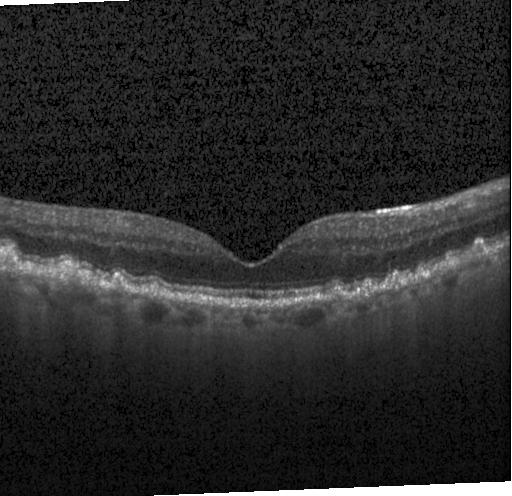 OCT line scan, fovea-centered.
Impression: multiple drusen.